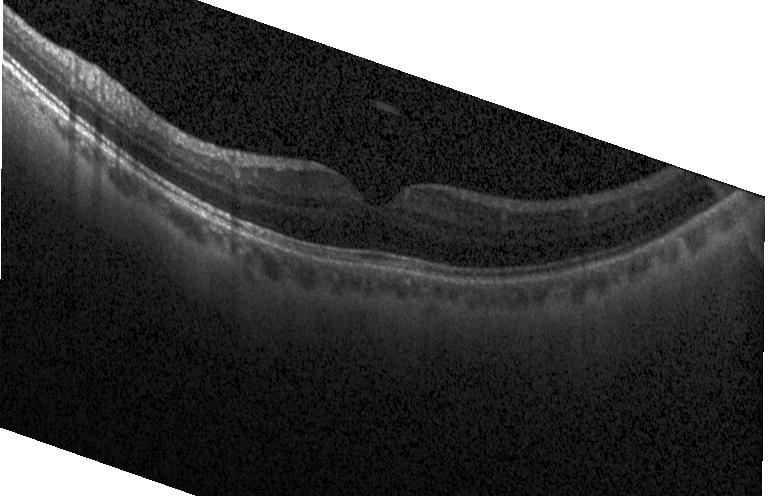
Acquired on a Heidelberg Spectralis. OCT line scan. Horizontal scan through the fovea — Diagnosis: no CNV, DME, or drusen.